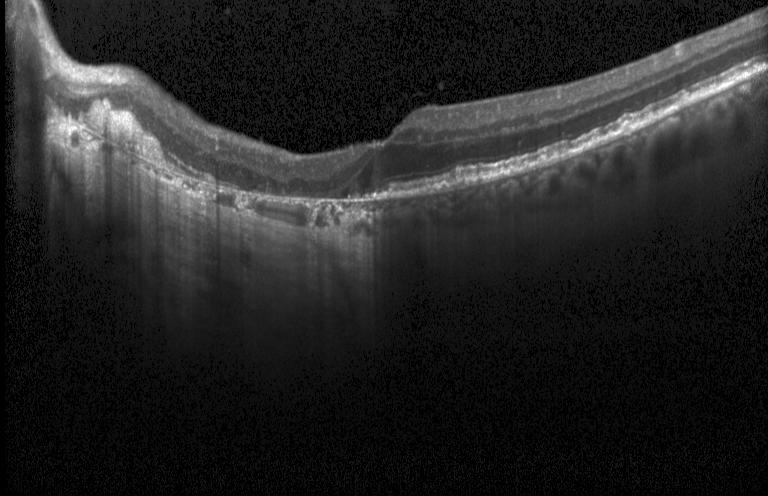 Dx: a choroidal neovascular membrane.